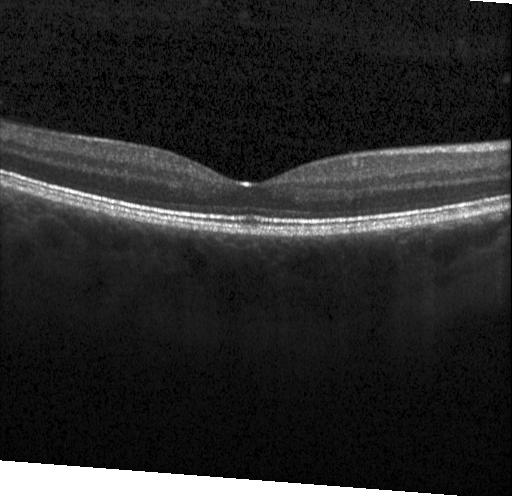 Optical coherence tomography B-scan. Spectral-domain optical coherence tomography. Acquired on a Heidelberg Spectralis. No choroidal neovascularization, diabetic macular edema, or drusen.